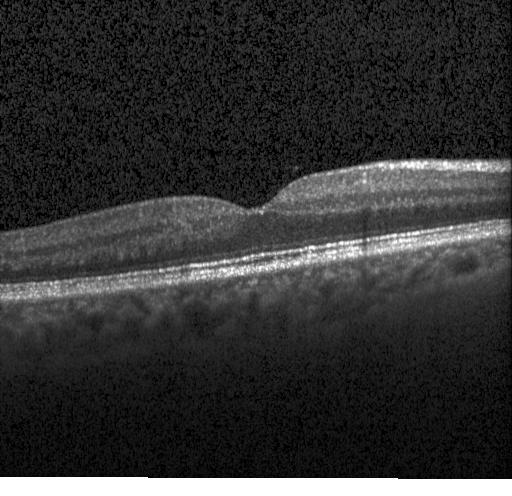 Finding: neither choroidal neovascularization, diabetic macular edema, nor drusen.